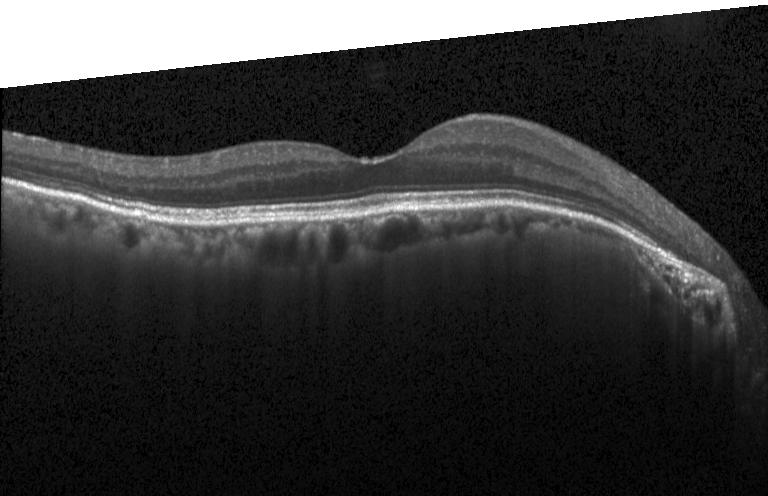 Impression: no evidence of choroidal neovascularization, diabetic macular edema, or drusen.